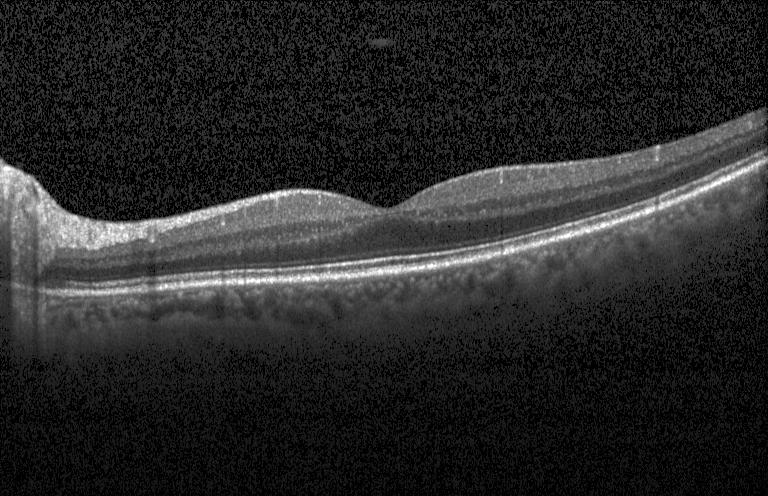
SD-OCT. Instrument: Heidelberg Spectralis. OCT line scan — Impression: neither choroidal neovascularization, diabetic macular edema, nor drusen.